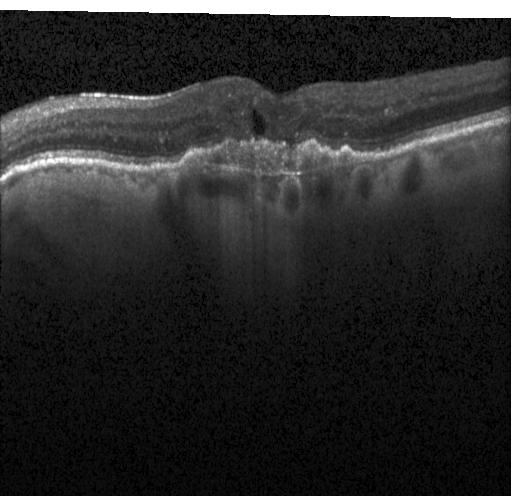

OCT B-scan.
Macular OCT: choroidal neovascularization.